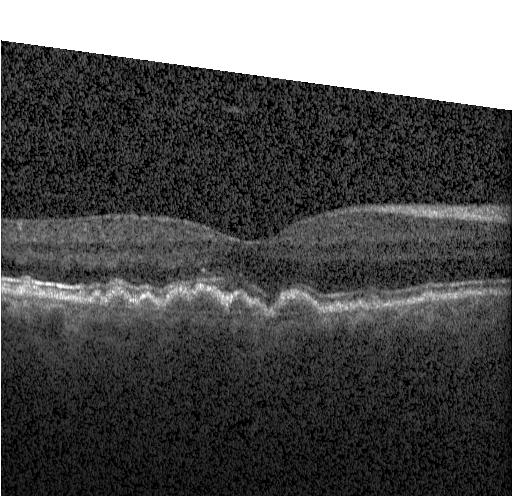

Retinal OCT cross-section, through the macula, spectral-domain OCT, Heidelberg Spectralis
Assessment: drusen.